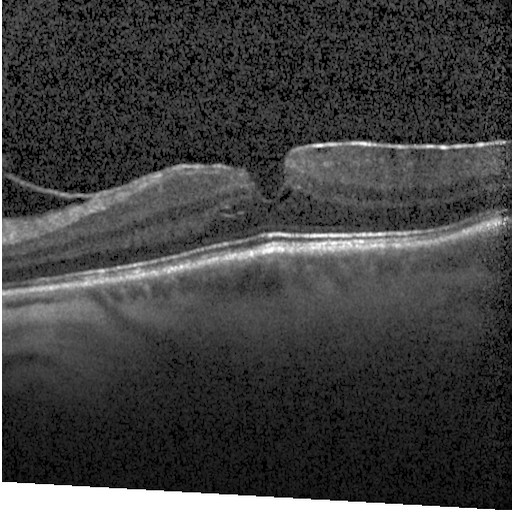
Horizontal scan through the fovea; retinal OCT cross-section. Diagnosis: diabetic macular edema.